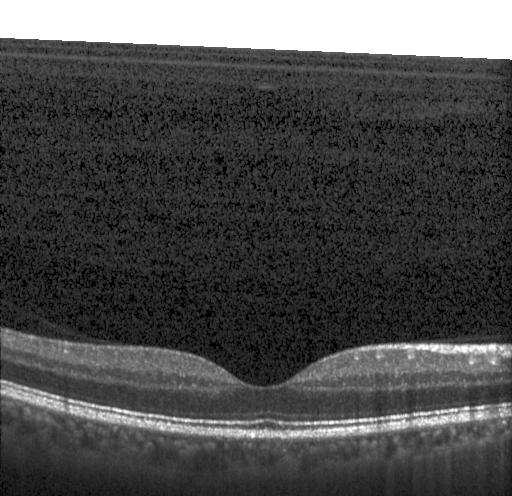
The scan shows no choroidal neovascularization, diabetic macular edema, or drusen.